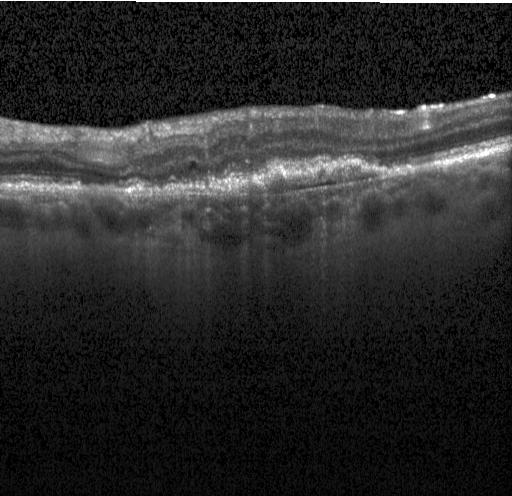 The scan shows choroidal neovascularization (CNV).